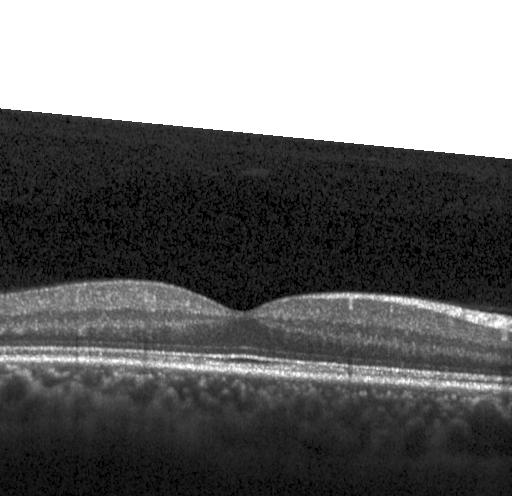
SD-OCT; horizontal scan through the fovea; retinal OCT cross-section. Impression: no CNV, DME, or drusen.